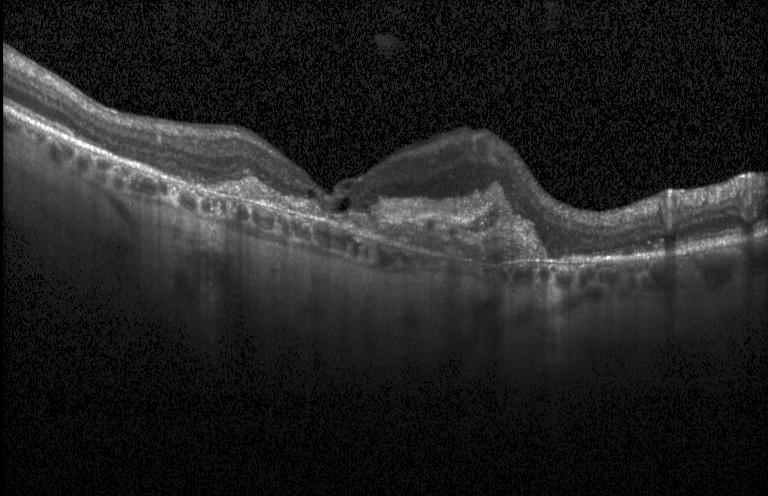

SD-OCT. Optical coherence tomography scan. Acquired on a Heidelberg Spectralis. Macular scan — This B-scan demonstrates a choroidal neovascular membrane.